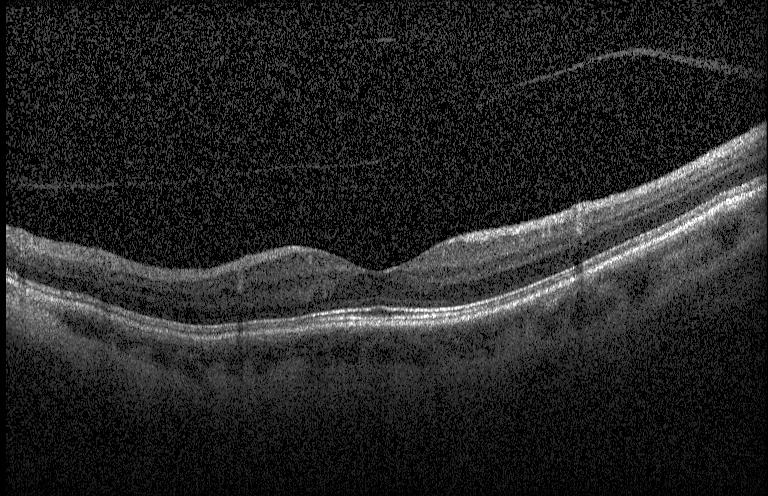 Retinal OCT cross-section showing neither choroidal neovascularization, diabetic macular edema, nor drusen.